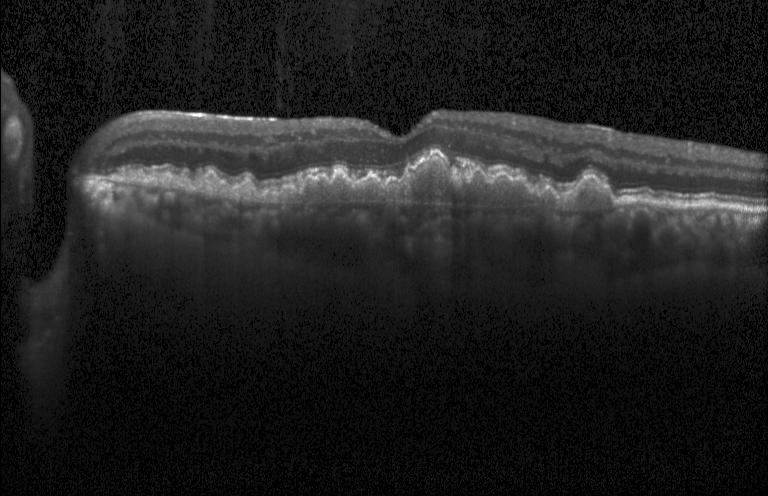
Retinal OCT B-scan. Diagnosis: choroidal neovascularization (CNV).